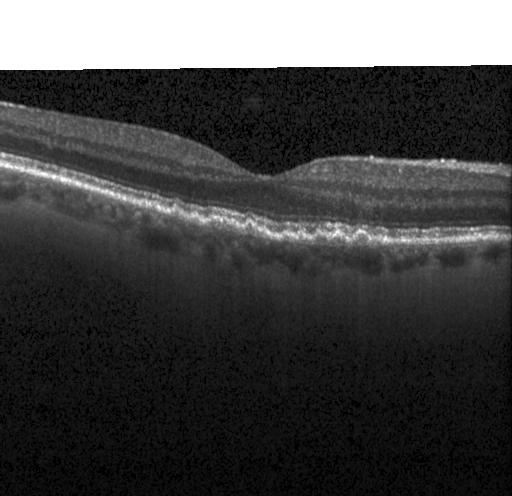 Diagnosis: drusen.